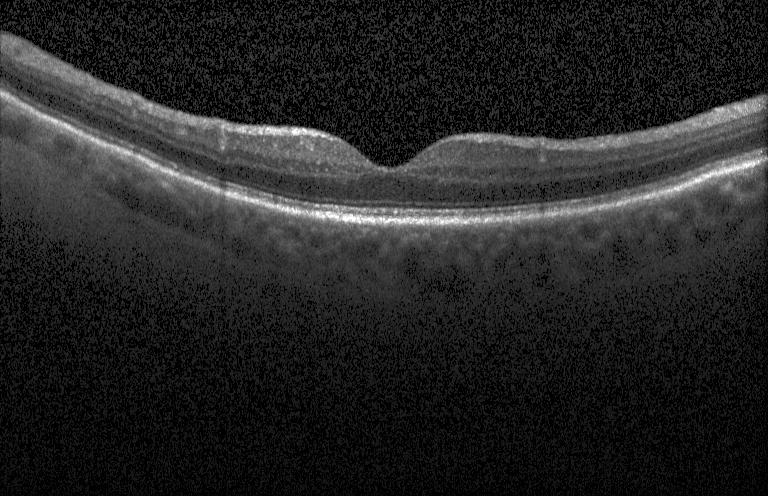 No CNV, DME, or drusen.